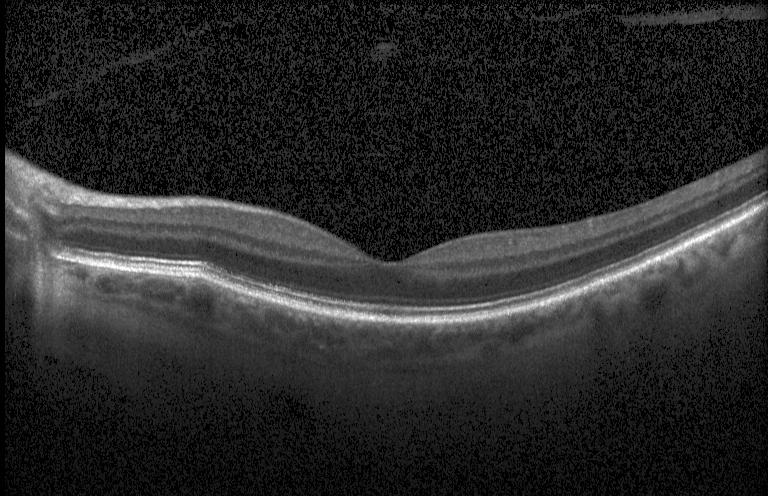

Neither choroidal neovascularization, diabetic macular edema, nor drusen.